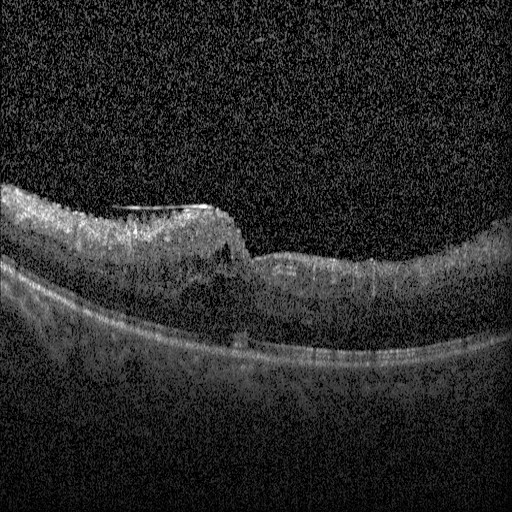 Spectral-domain OCT · retinal OCT B-scan · through the macula.
Impression: DME.